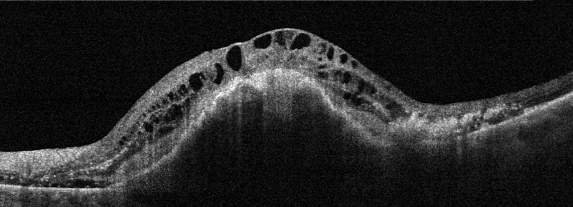

Finding: AMD.